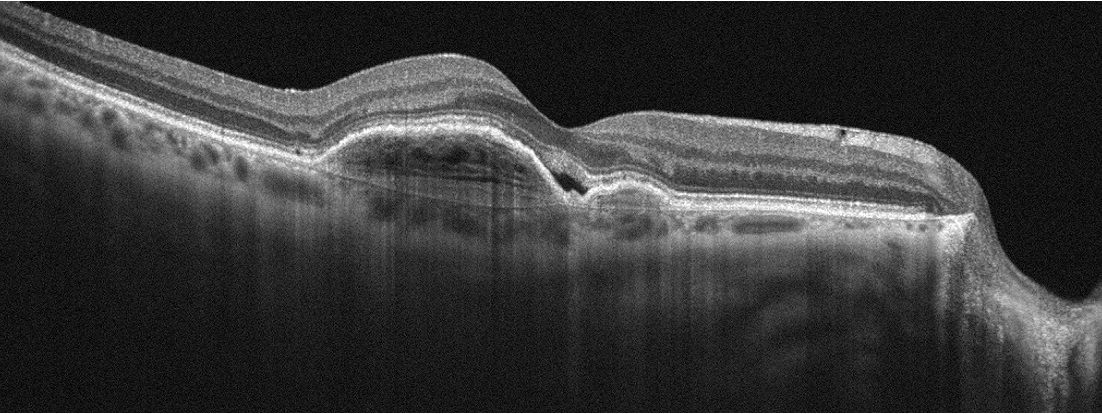 Optical coherence tomography B-scan · Optovue Avanti RTVue XR — The scan shows AMD.